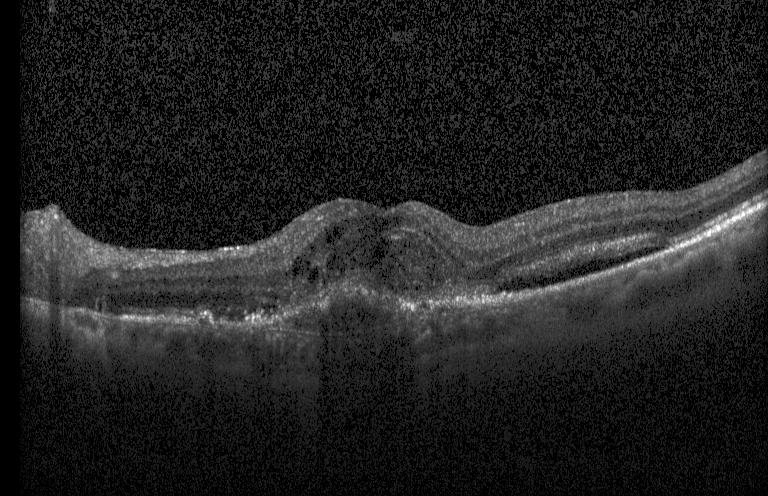

Diagnosis: a choroidal neovascular membrane.